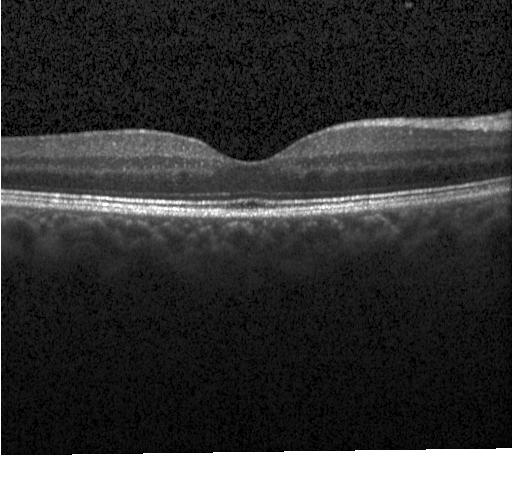 SD-OCT, acquired on a Heidelberg Spectralis, macular scan, optical coherence tomography scan. Macular OCT: no choroidal neovascularization, diabetic macular edema, or drusen.